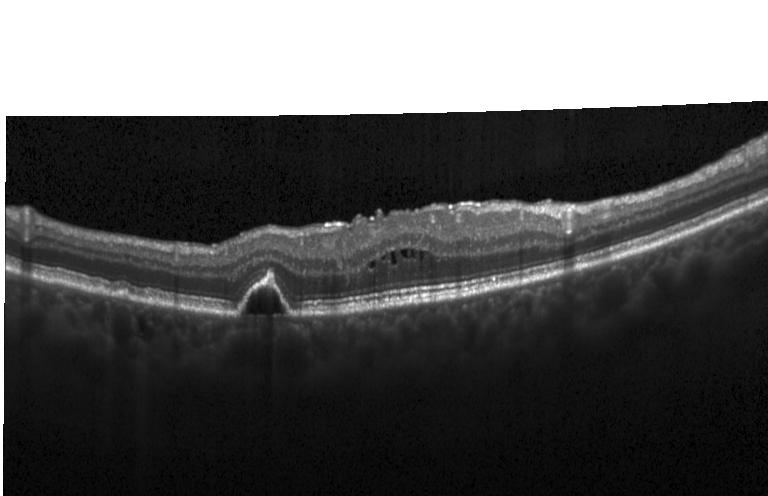 Spectral-domain OCT; retinal OCT B-scan.
A choroidal neovascular membrane.